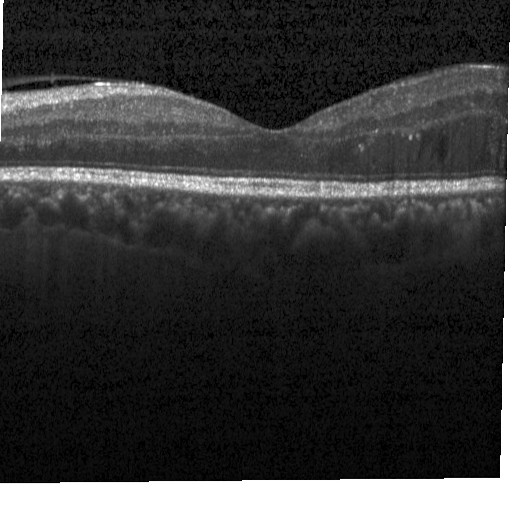
Finding: diabetic macular edema.